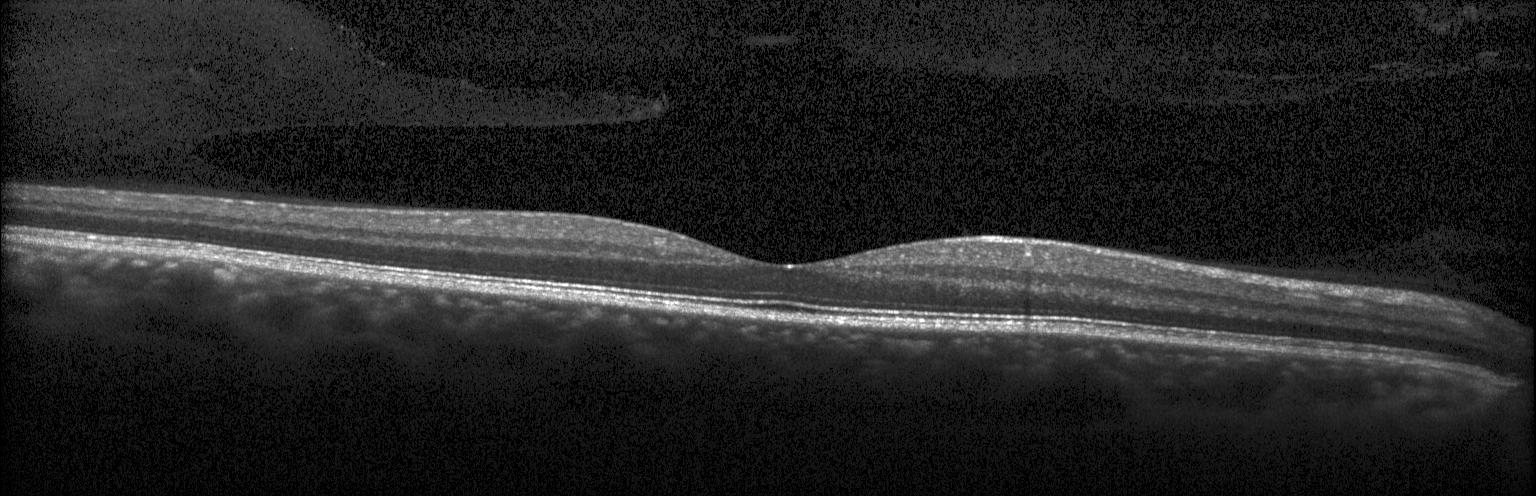

Optical coherence tomography scan · acquired on a Heidelberg Spectralis. Diagnosis: neither choroidal neovascularization, diabetic macular edema, nor drusen.